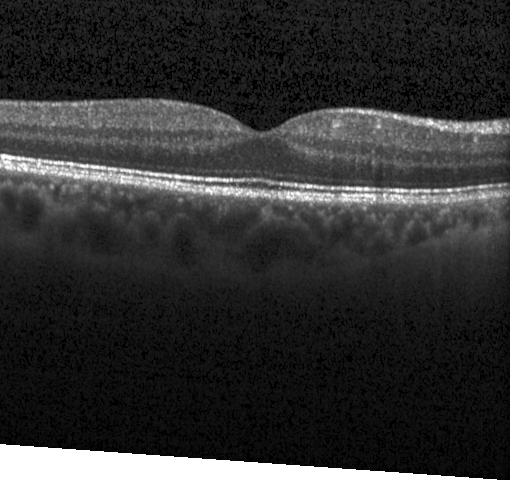
Optical coherence tomography B-scan; centered on the fovea; instrument: Heidelberg Spectralis. This B-scan demonstrates no choroidal neovascularization, no diabetic macular edema, and no drusen.